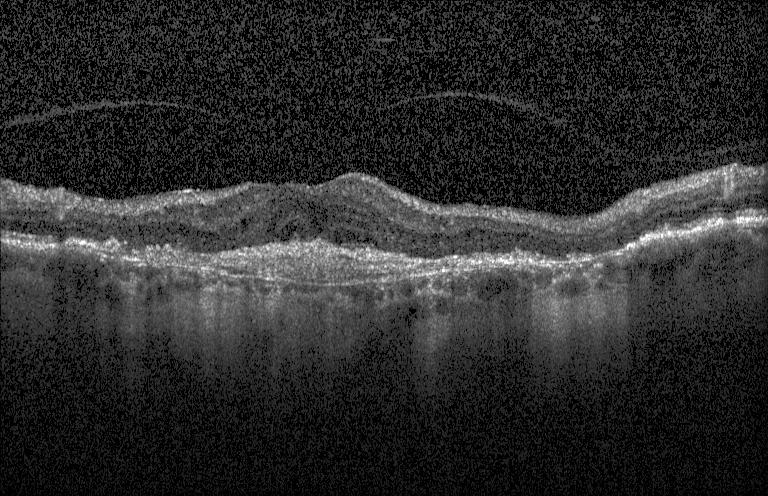

Spectral-domain OCT B-scan: choroidal neovascularization (CNV).